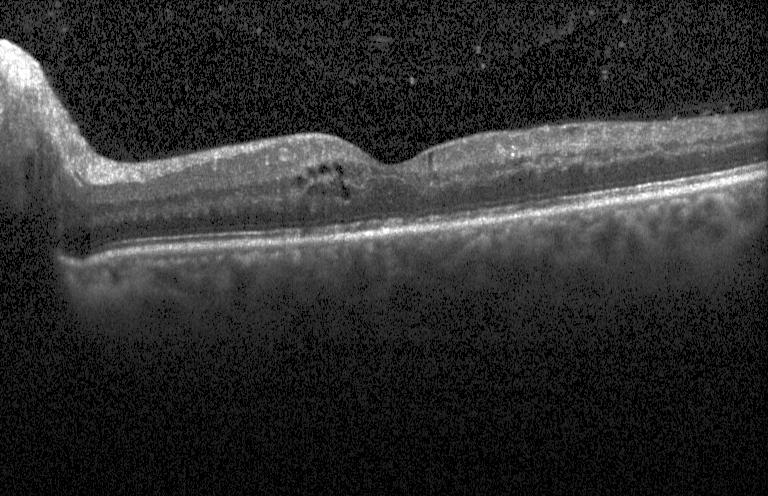

Macular scan, spectral-domain optical coherence tomography, acquired on a Heidelberg Spectralis, retinal OCT B-scan.
Assessment: diabetic macular edema.